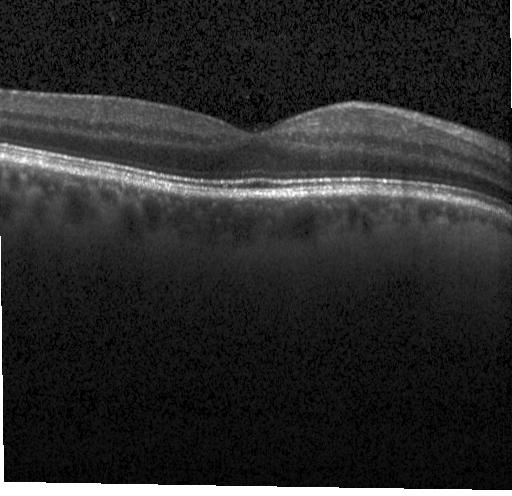
Optical coherence tomography B-scan. Heidelberg Spectralis OCT system. Macular scan — Impression: neither choroidal neovascularization, diabetic macular edema, nor drusen.